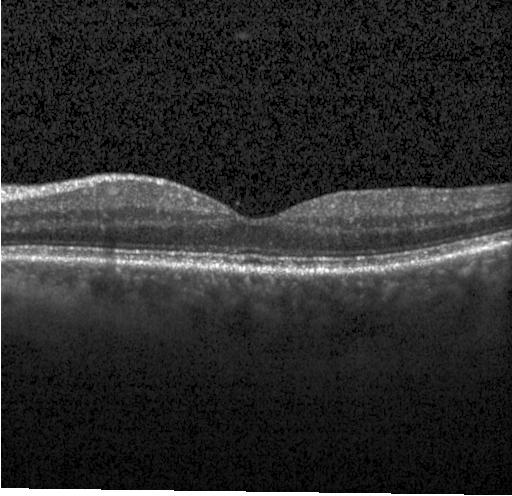

OCT line scan, instrument: Heidelberg Spectralis, spectral-domain optical coherence tomography, fovea-centered — Impression: no choroidal neovascularization, no diabetic macular edema, and no drusen.